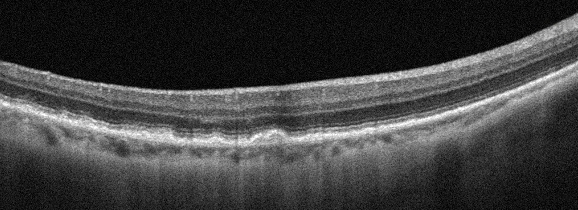
Right eye. Retinal OCT cross-section
Age-related macular degeneration.